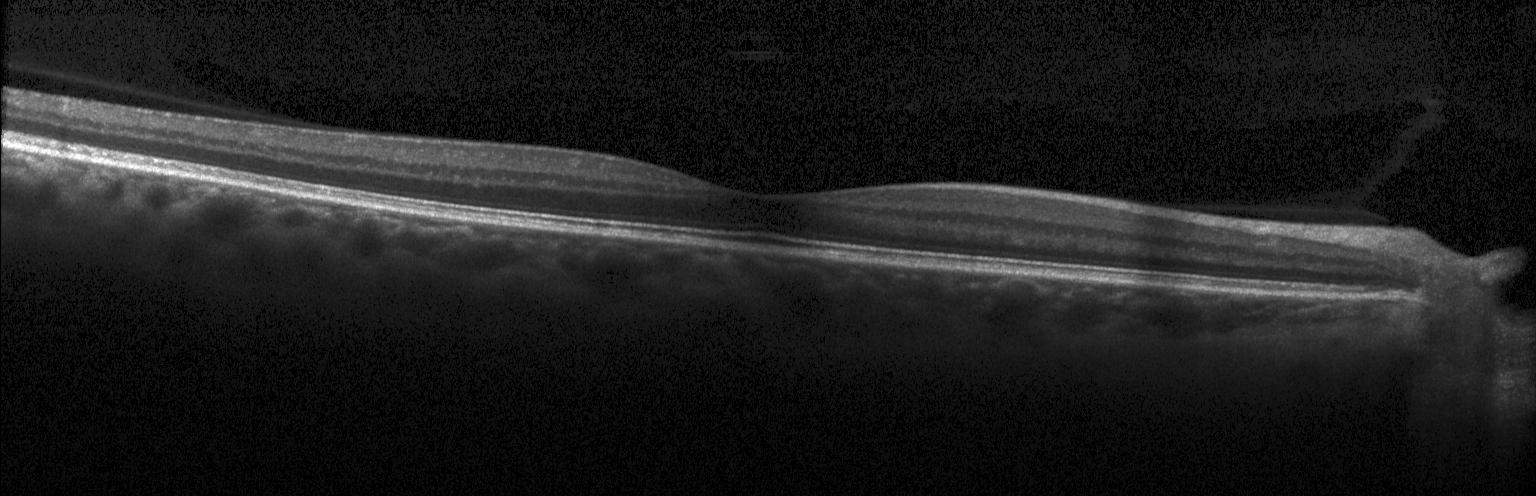
OCT finding: neither choroidal neovascularization, diabetic macular edema, nor drusen.